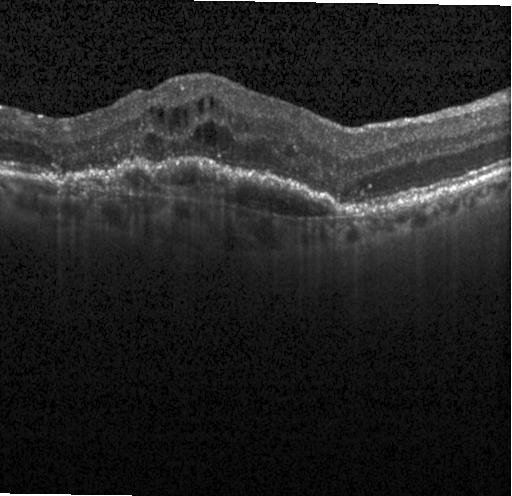
Heidelberg Spectralis OCT system, retinal OCT B-scan, horizontal scan through the fovea. Assessment: a choroidal neovascular membrane.